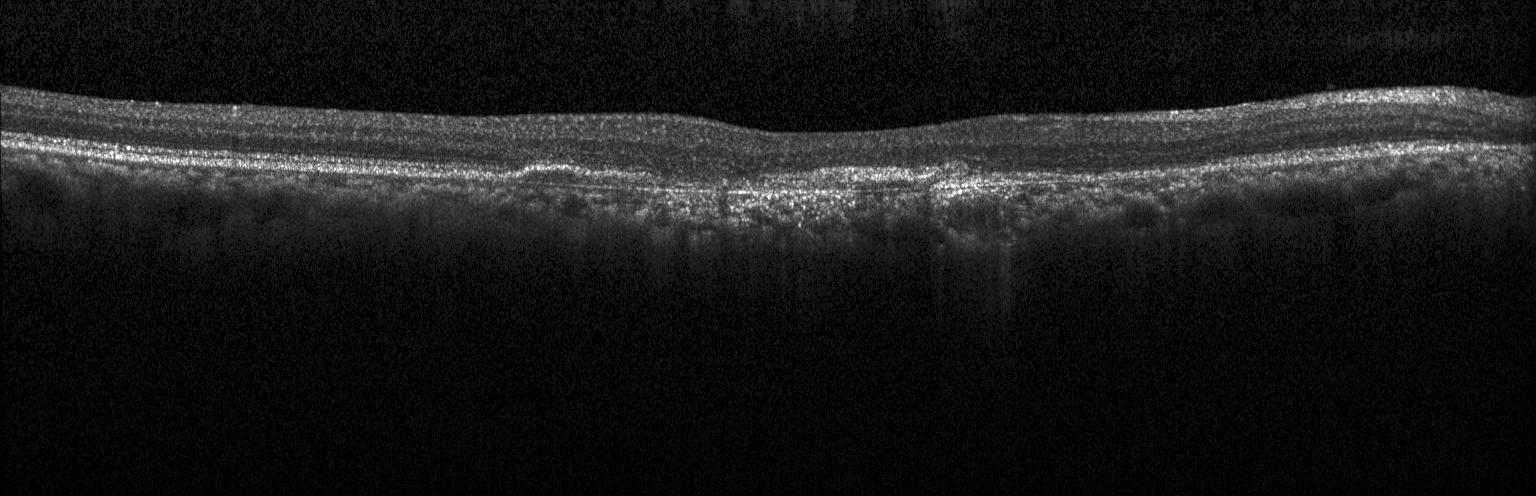

Optical coherence tomography scan. Horizontal scan through the fovea. Instrument: Heidelberg Spectralis. Macular OCT: choroidal neovascularization (CNV).